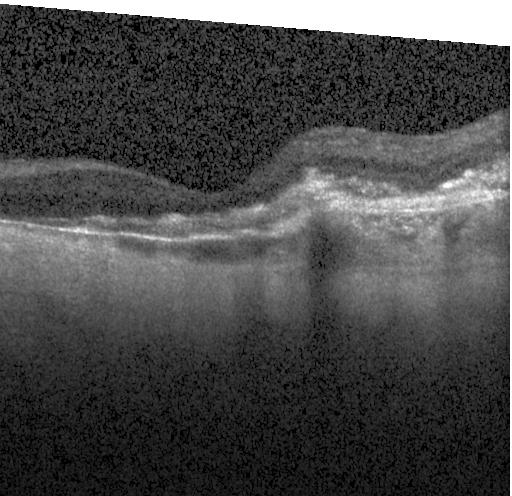 Retinal OCT cross-section; instrument: Heidelberg Spectralis — Macular OCT: a choroidal neovascular membrane.